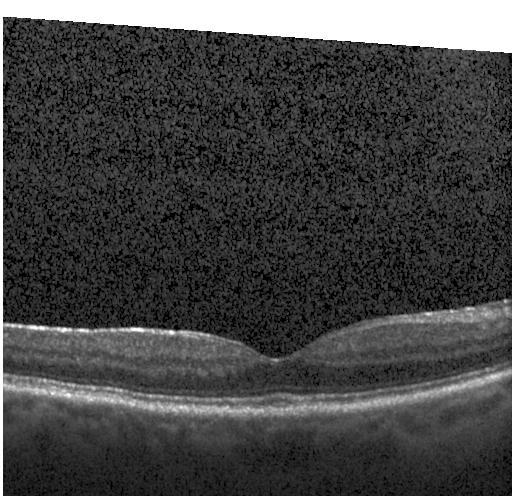

OCT line scan; spectral-domain optical coherence tomography; through the macula. The scan shows neither choroidal neovascularization, diabetic macular edema, nor drusen.